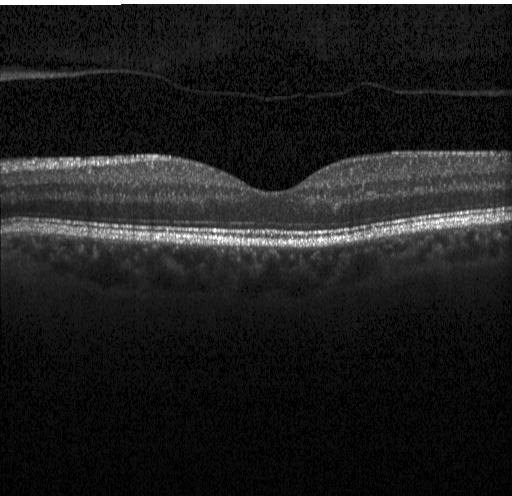
Instrument: Heidelberg Spectralis. OCT line scan.
Neither CNV, DME, nor drusen.